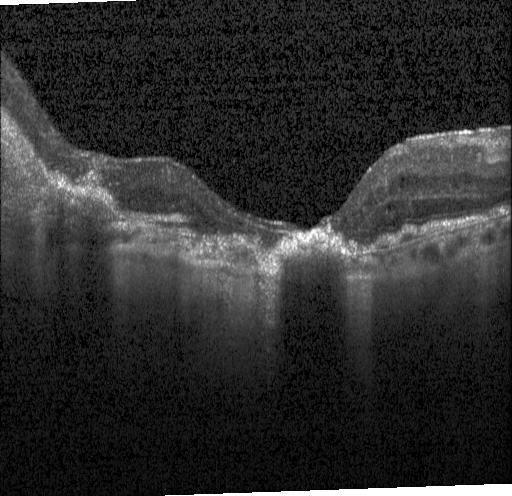 Horizontal scan through the fovea · spectral-domain optical coherence tomography · OCT line scan · acquired on a Heidelberg Spectralis — This B-scan demonstrates choroidal neovascularization.